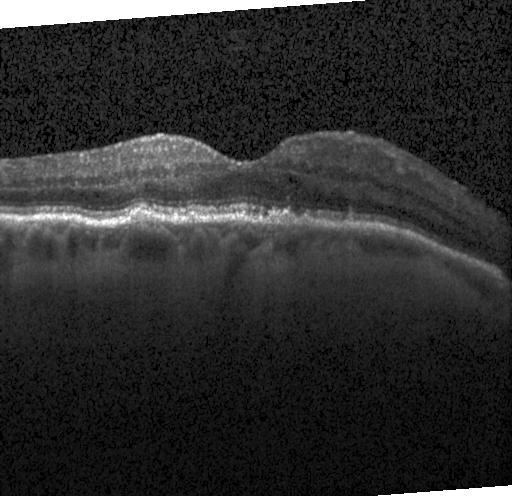
Dx: a choroidal neovascular membrane.